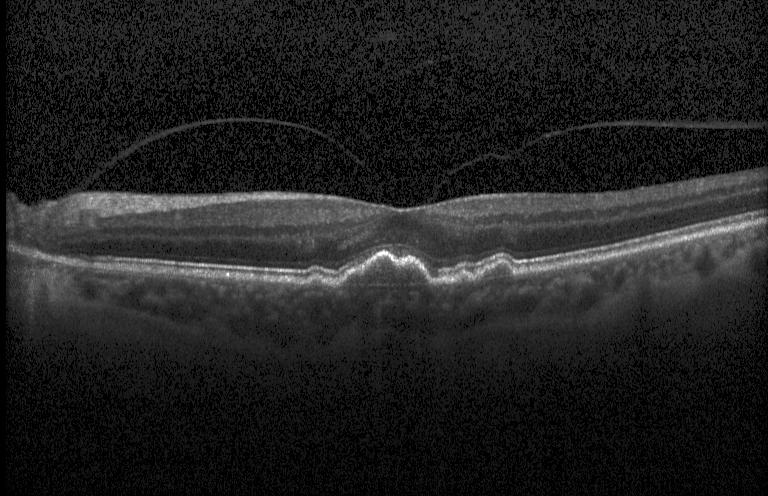

Macular scan, OCT line scan, Heidelberg Spectralis OCT system, SD-OCT. Impression: drusen.